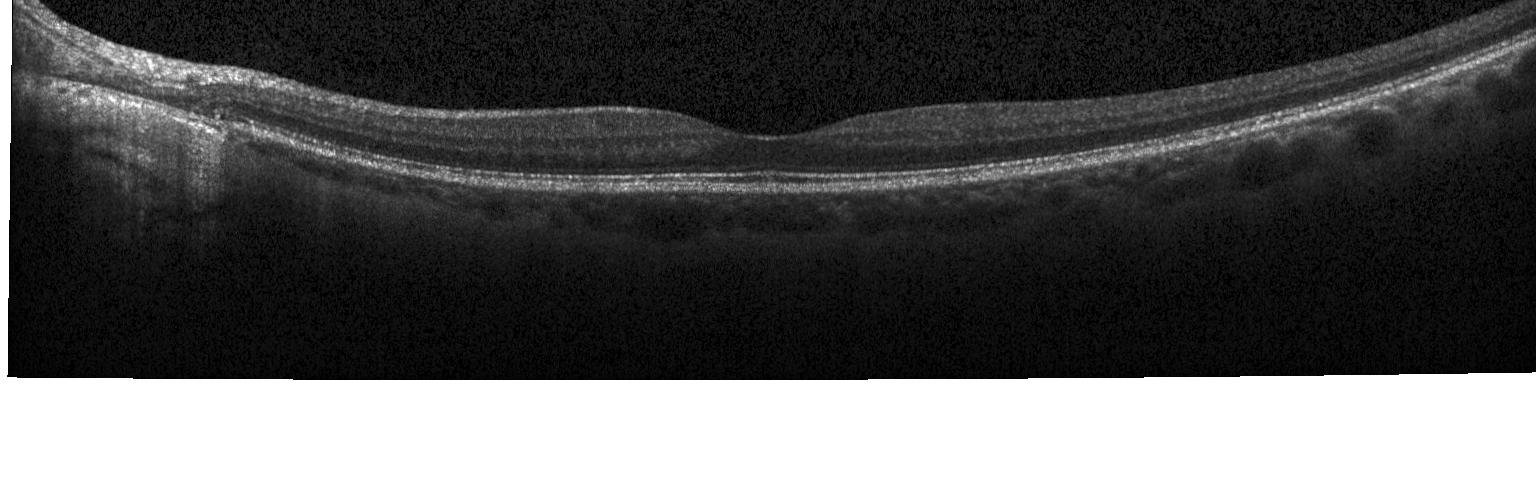

Macular OCT demonstrating no choroidal neovascularization, no diabetic macular edema, and no drusen.